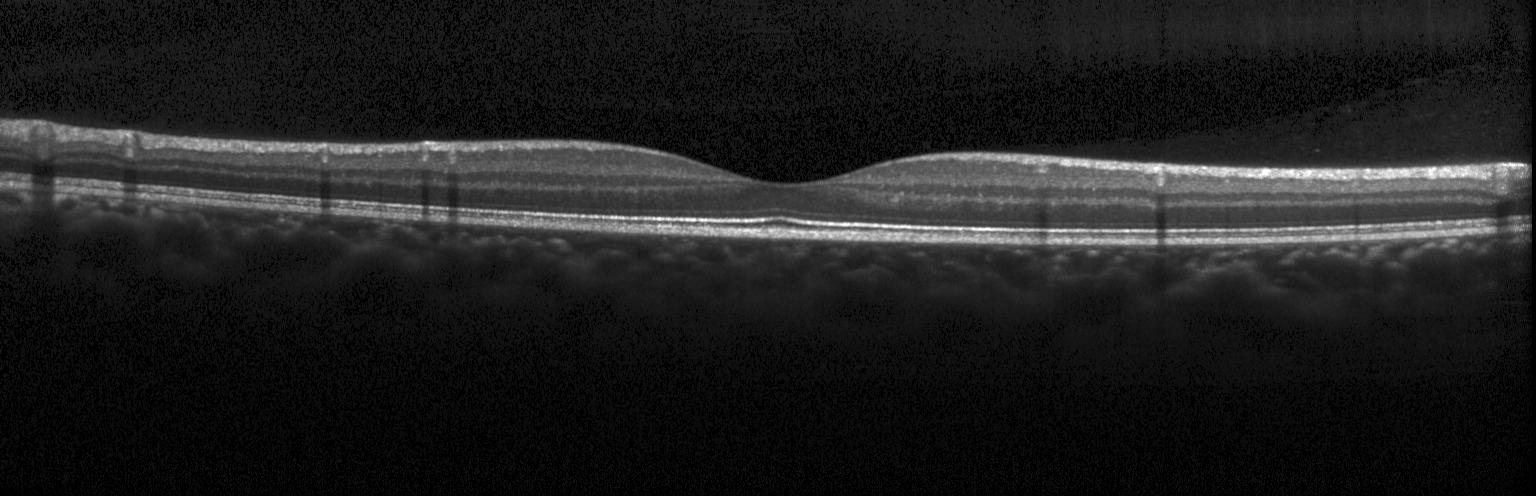

Optical coherence tomography B-scan.
Finding: neither choroidal neovascularization, diabetic macular edema, nor drusen.